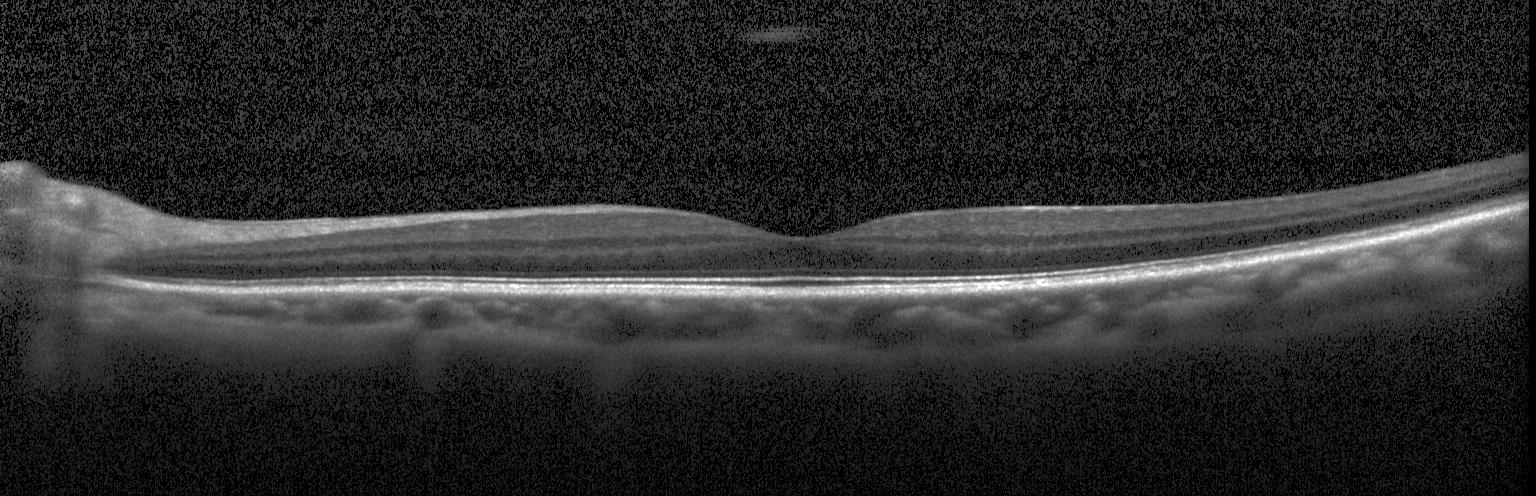 Retinal OCT cross-section
Macular OCT: no choroidal neovascularization, no diabetic macular edema, and no drusen.